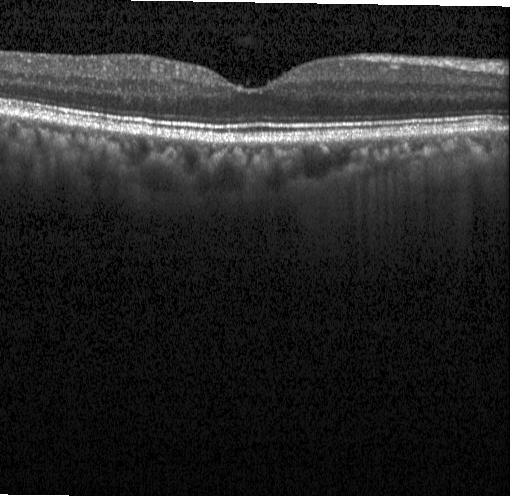
SD-OCT. Optical coherence tomography B-scan
Assessment: no choroidal neovascularization, no diabetic macular edema, and no drusen.